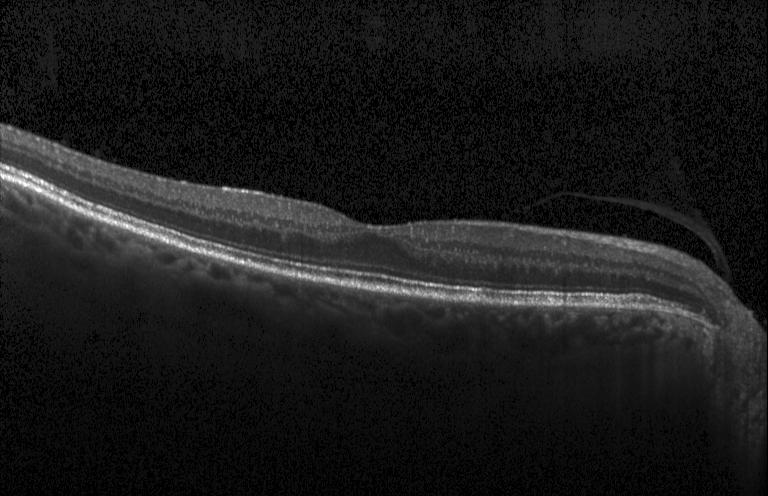 Finding: neither CNV, DME, nor drusen.